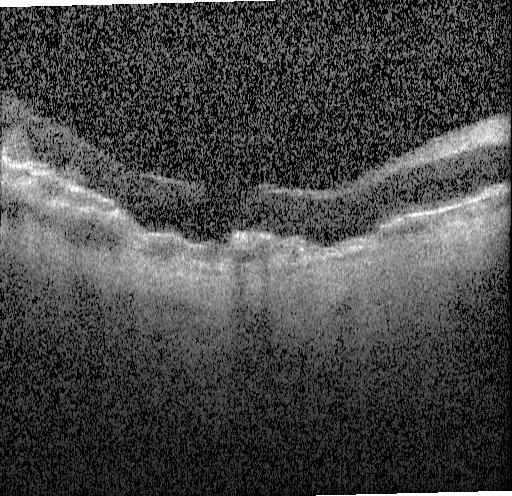

Spectral-domain OCT, Heidelberg Spectralis, optical coherence tomography scan — The scan shows CNV.